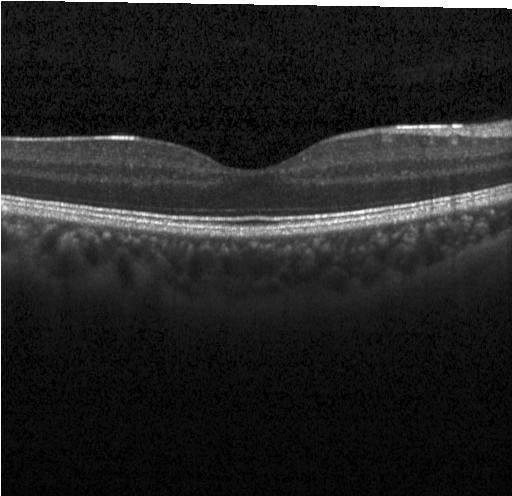 Macular scan, OCT B-scan, SD-OCT
Assessment: no CNV, no DME, and no drusen.